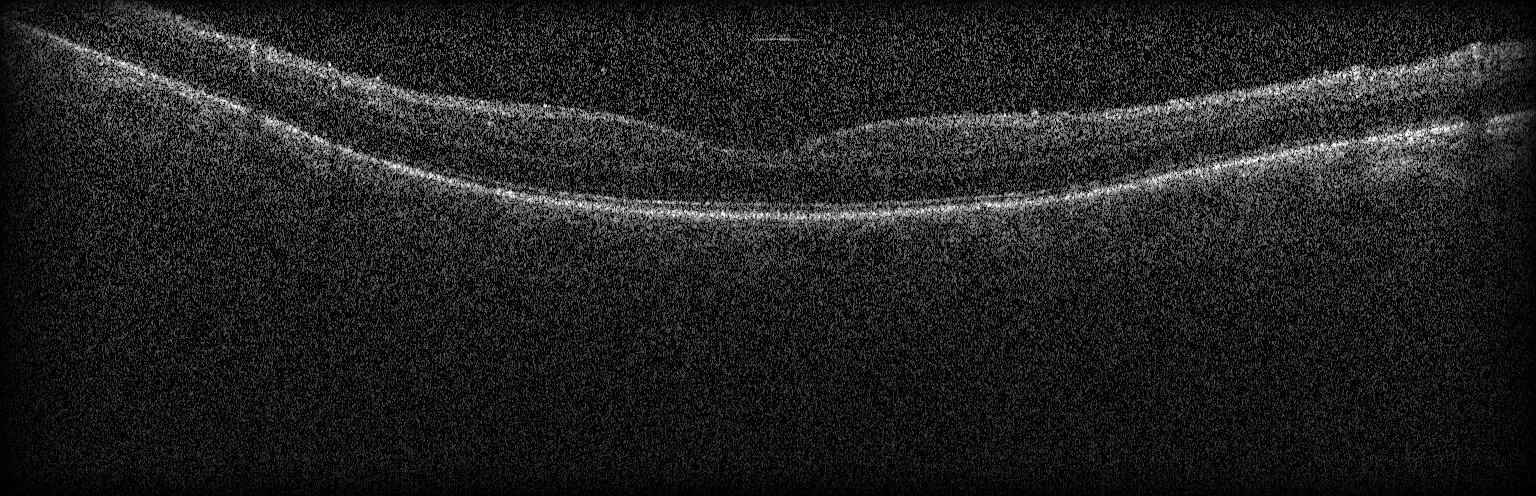
Retinal OCT cross-section showing no evidence of choroidal neovascularization, diabetic macular edema, or drusen.